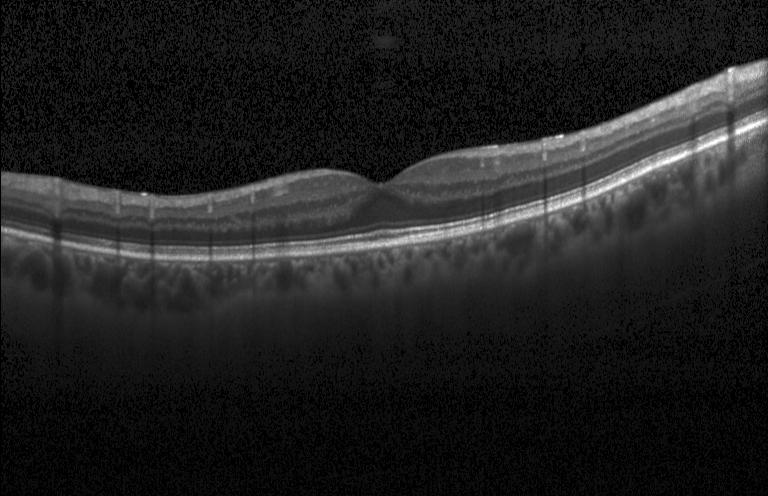
Optical coherence tomography B-scan, macular scan, spectral-domain OCT, Heidelberg Spectralis. OCT finding: no evidence of CNV, DME, or drusen.